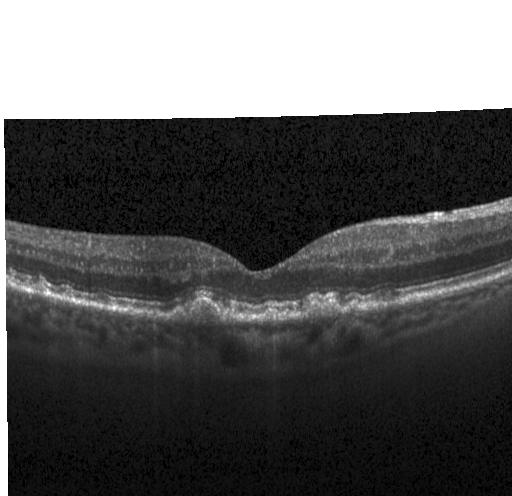
Macular OCT demonstrating multiple drusen.